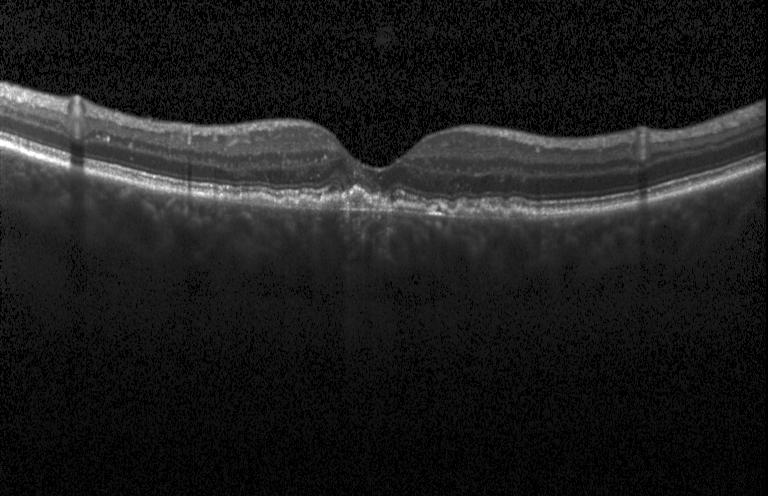 This B-scan demonstrates a choroidal neovascular membrane.